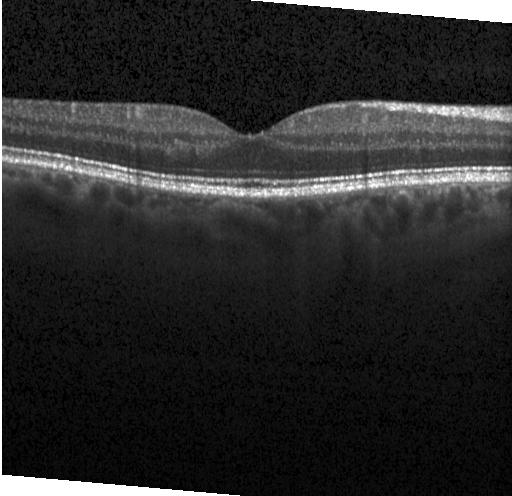

OCT B-scan; acquired on a Heidelberg Spectralis
The scan shows no evidence of choroidal neovascularization, diabetic macular edema, or drusen.